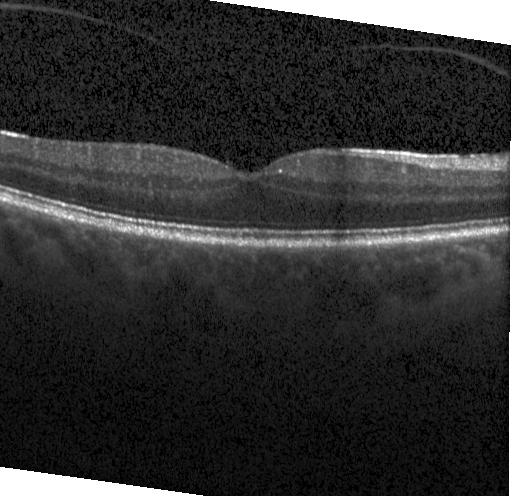

Retinal OCT cross-section · spectral-domain optical coherence tomography.
No evidence of choroidal neovascularization, diabetic macular edema, or drusen.